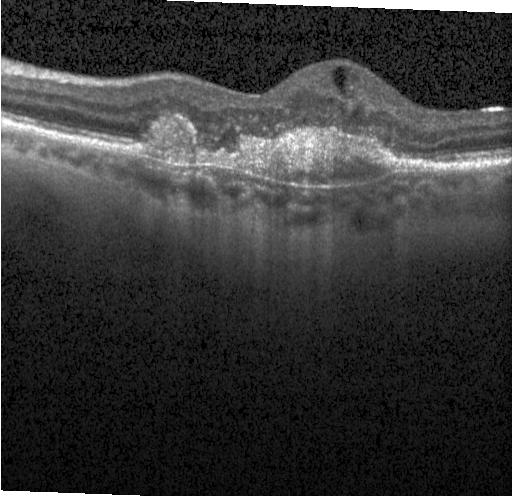
OCT line scan. Through the macula — A choroidal neovascular membrane.